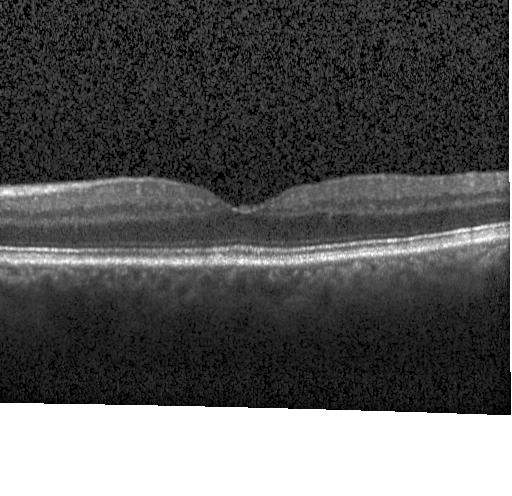

Retinal OCT cross-section. Instrument: Heidelberg Spectralis — Neither CNV, DME, nor drusen.